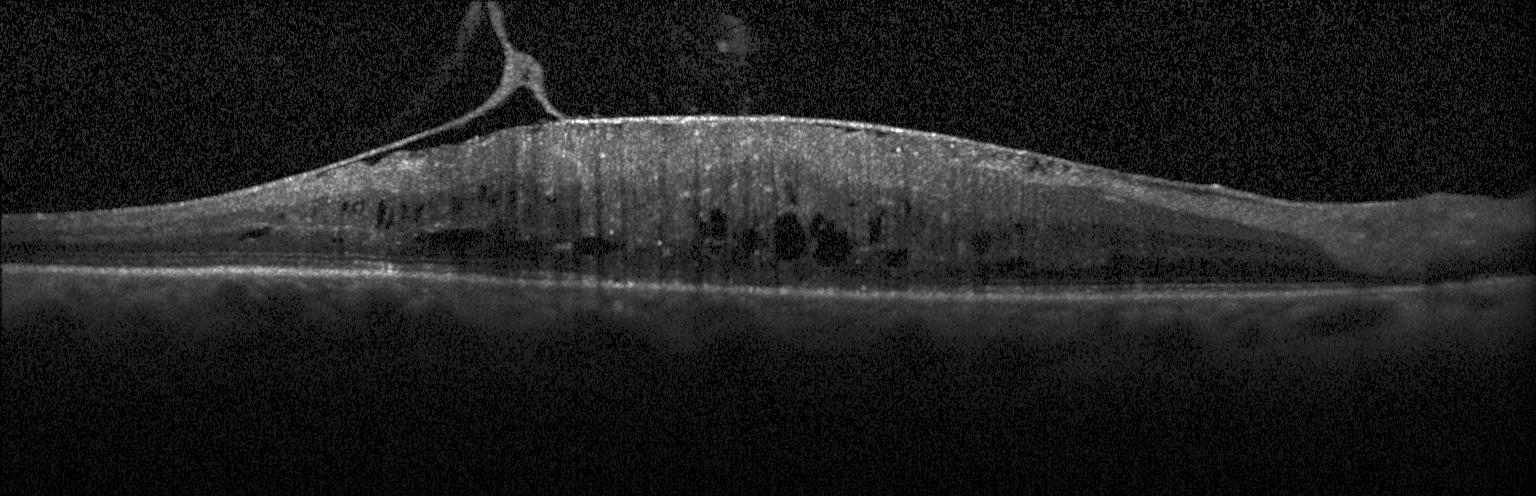

Impression: DME.